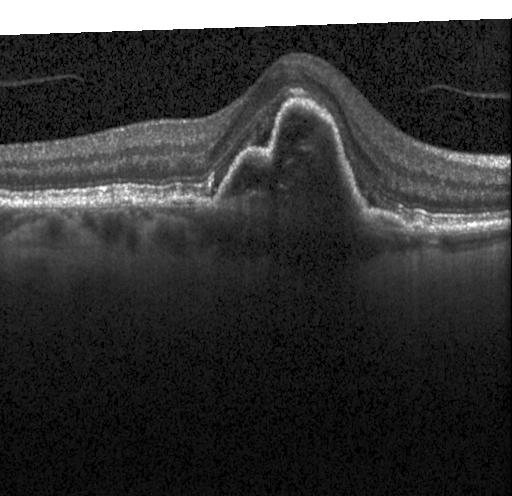

Retinal OCT B-scan.
Impression: a choroidal neovascular membrane.